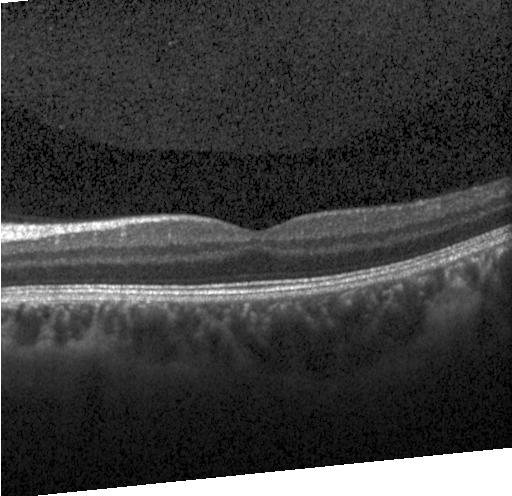
Retinal OCT B-scan
Finding: no evidence of CNV, DME, or drusen.